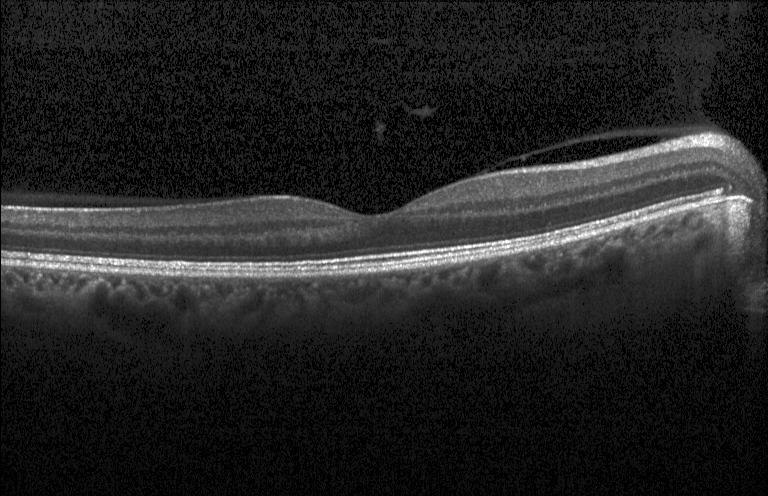 The scan shows no evidence of choroidal neovascularization, diabetic macular edema, or drusen.